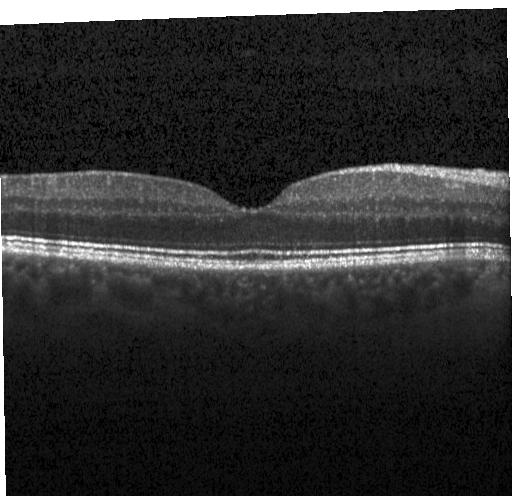

Optical coherence tomography B-scan — This B-scan demonstrates neither choroidal neovascularization, diabetic macular edema, nor drusen.